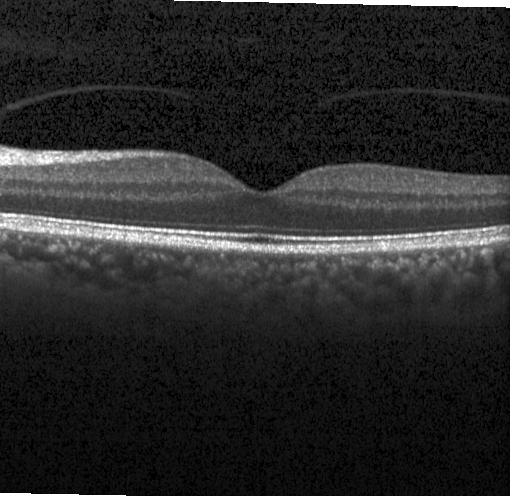 OCT finding: neither choroidal neovascularization, diabetic macular edema, nor drusen.